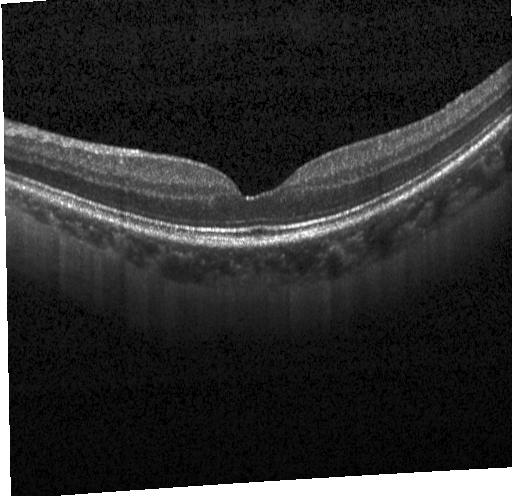

Horizontal scan through the fovea, acquired on a Heidelberg Spectralis, retinal OCT B-scan — No CNV, no DME, and no drusen.